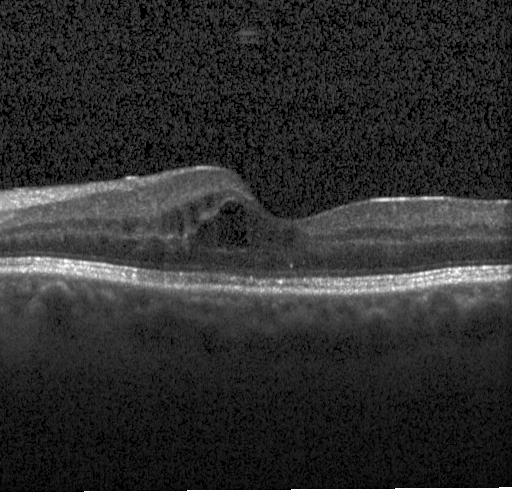 Optical coherence tomography scan; horizontal scan through the fovea.
This B-scan demonstrates diabetic macular edema.